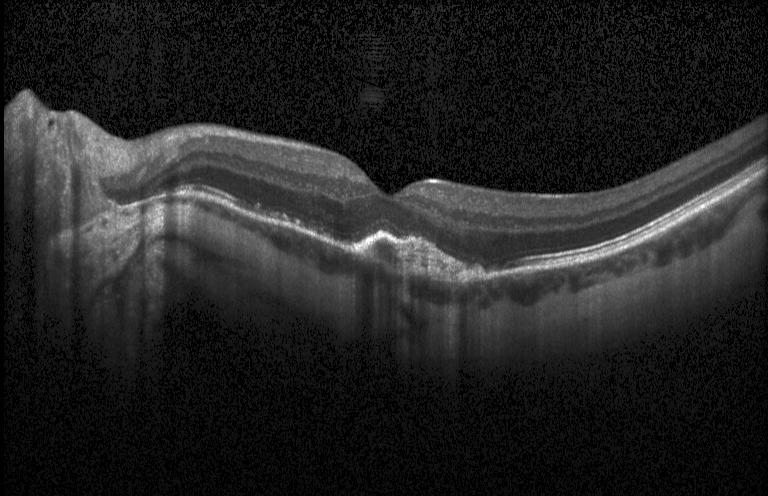

Acquired on a Heidelberg Spectralis. Retinal OCT B-scan
Dx: CNV.